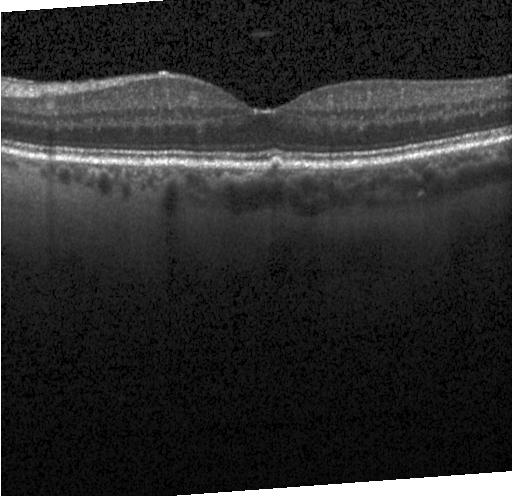 Optical coherence tomography B-scan.
Impression: sub-RPE drusenoid deposits.